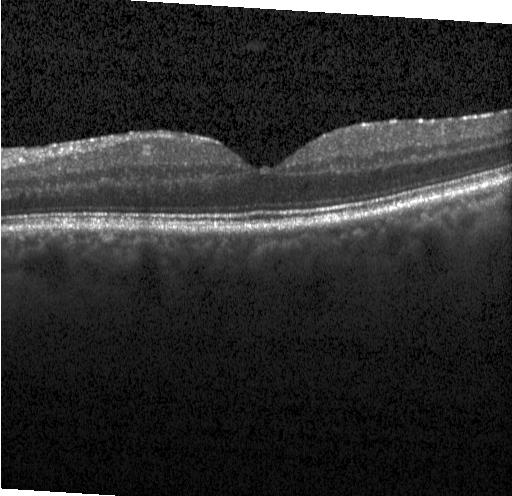

SD-OCT; retinal OCT cross-section — Impression: no choroidal neovascularization, no diabetic macular edema, and no drusen.